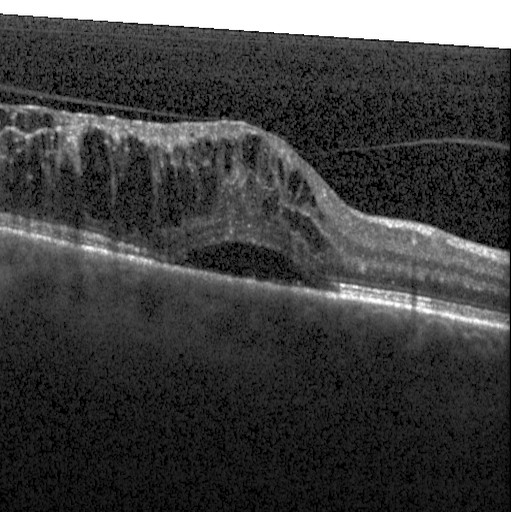

Optical coherence tomography scan, fovea-centered, spectral-domain OCT, acquired on a Heidelberg Spectralis. Diabetic macular edema.